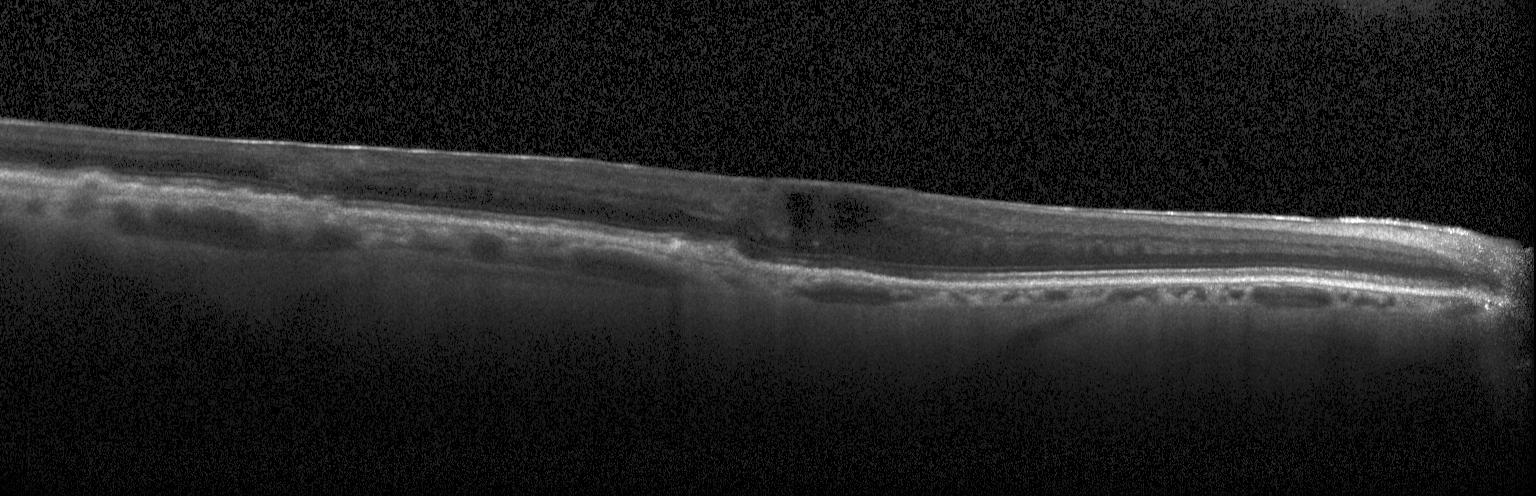

OCT line scan. Macular scan
Assessment: a choroidal neovascular membrane.